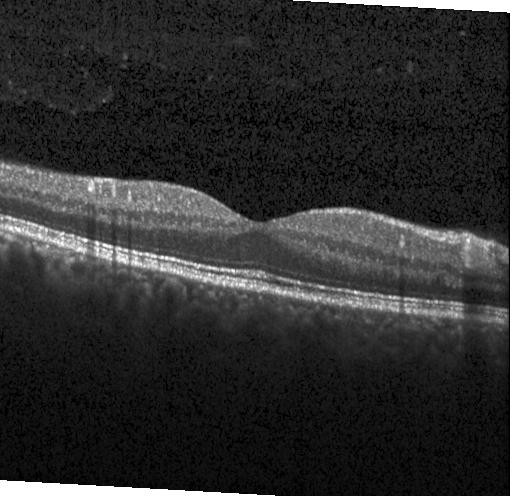 Retinal OCT cross-section
OCT finding: neither choroidal neovascularization, diabetic macular edema, nor drusen.